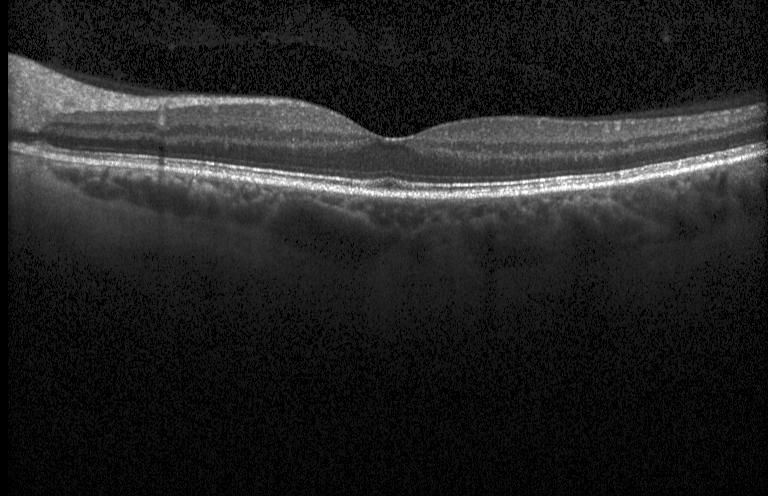
Impression: no evidence of choroidal neovascularization, diabetic macular edema, or drusen.